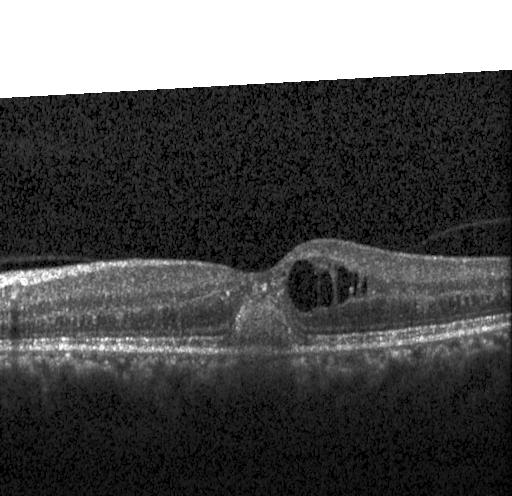
Spectral-domain optical coherence tomography, retinal OCT B-scan
Macular OCT: a choroidal neovascular membrane.